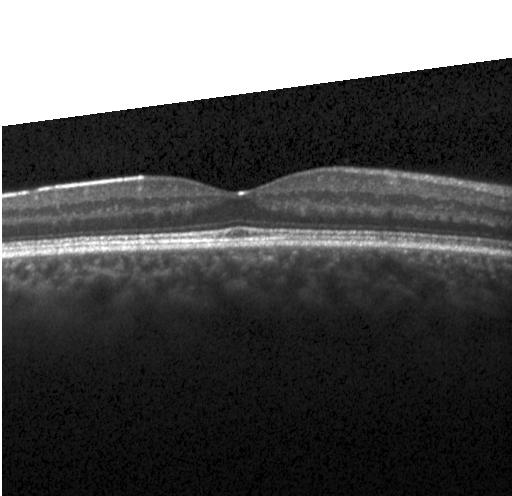
OCT B-scan — Assessment: neither CNV, DME, nor drusen.